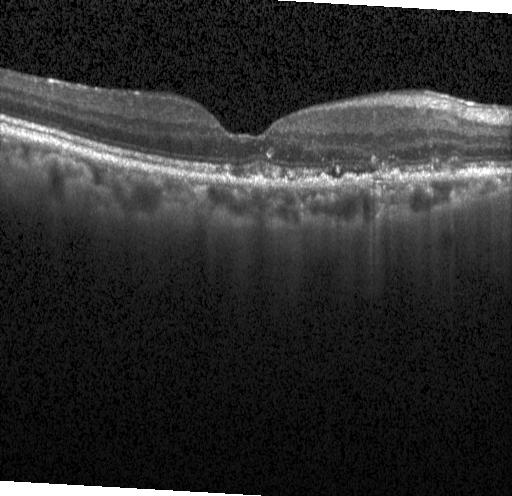 The scan shows choroidal neovascularization (CNV).